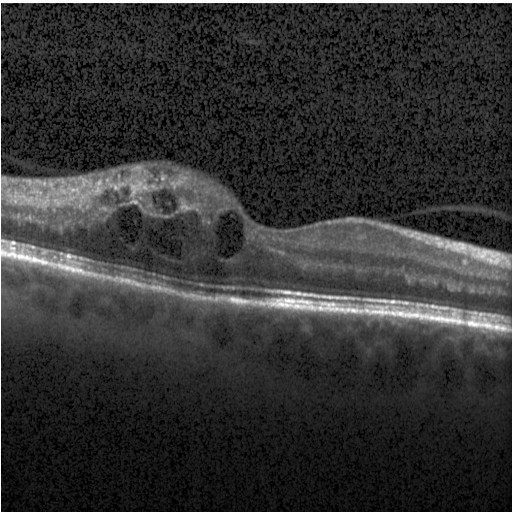

Retinal OCT B-scan; Heidelberg Spectralis; spectral-domain OCT; fovea-centered. Macular OCT: diabetic macular edema.